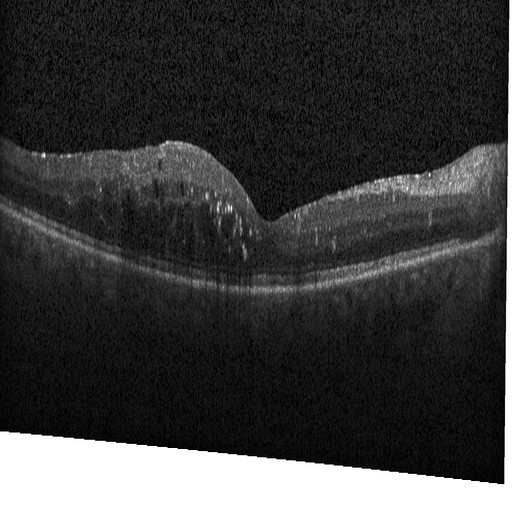

Optical coherence tomography B-scan.
Macular OCT: DME.